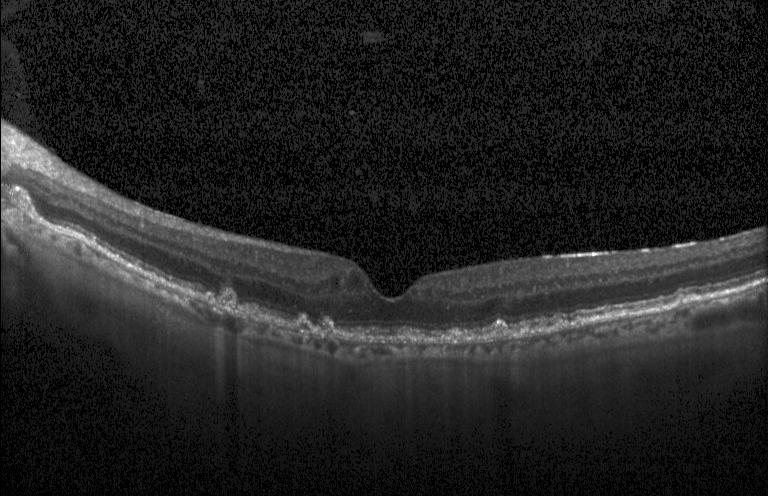
Impression: a choroidal neovascular membrane.